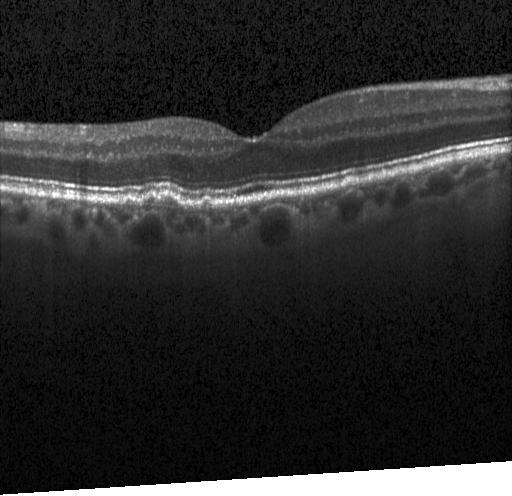
Optical coherence tomography B-scan.
Diagnosis: drusen.